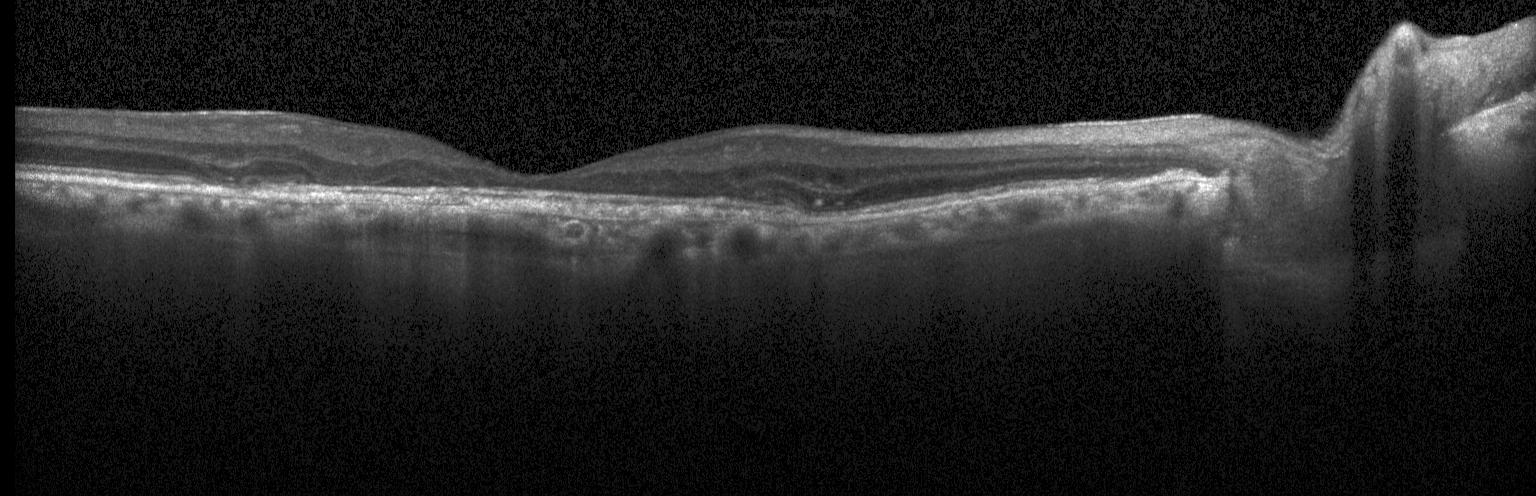 SD-OCT; OCT B-scan
A choroidal neovascular membrane.